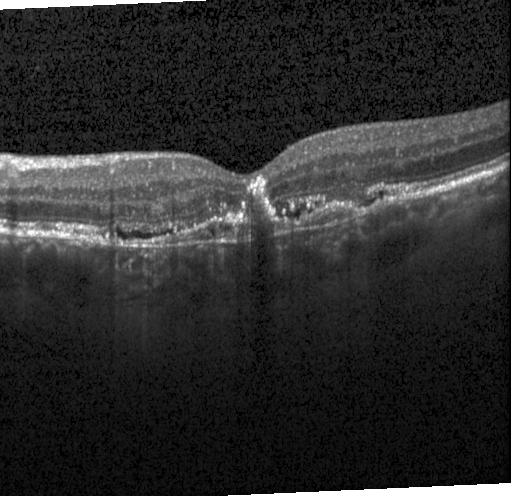
SD-OCT. Optical coherence tomography scan. Through the macula — Impression: a choroidal neovascular membrane.